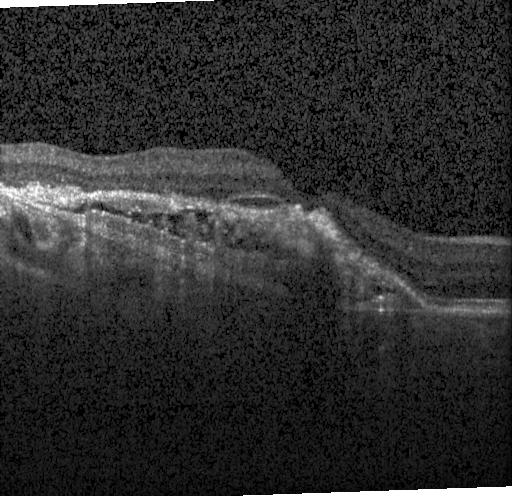
Retinal OCT cross-section. SD-OCT. Fovea-centered — Impression: CNV.